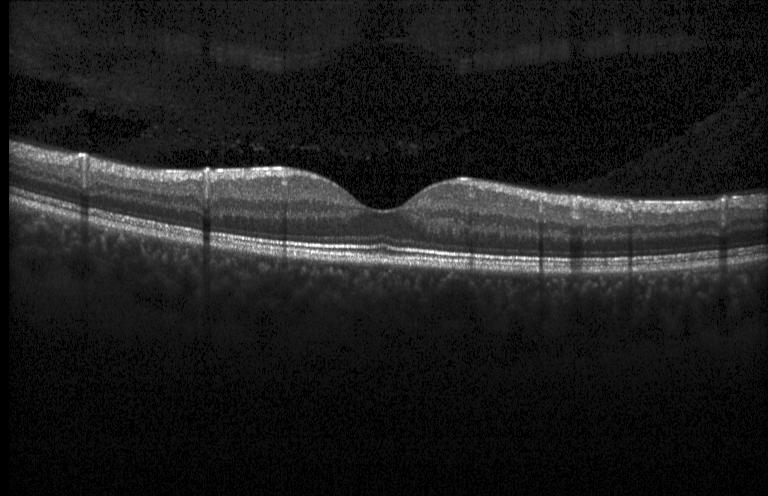

OCT B-scan showing no CNV, DME, or drusen.